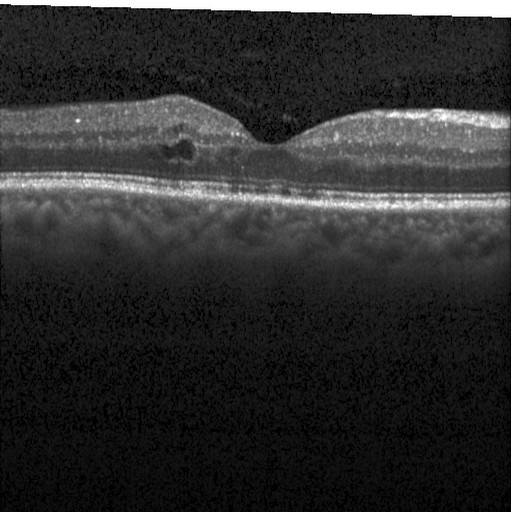 OCT finding: diabetic macular edema (DME).